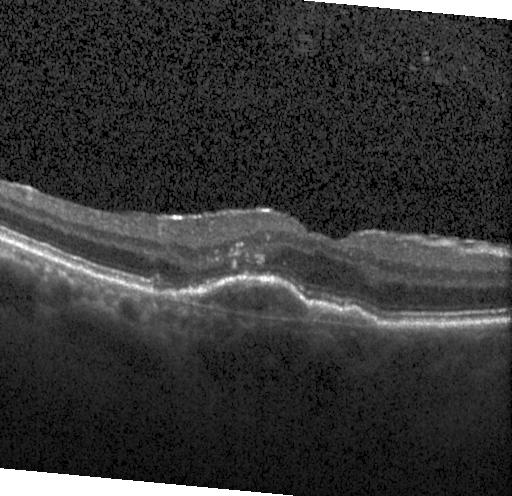

OCT line scan.
Impression: a choroidal neovascular membrane.